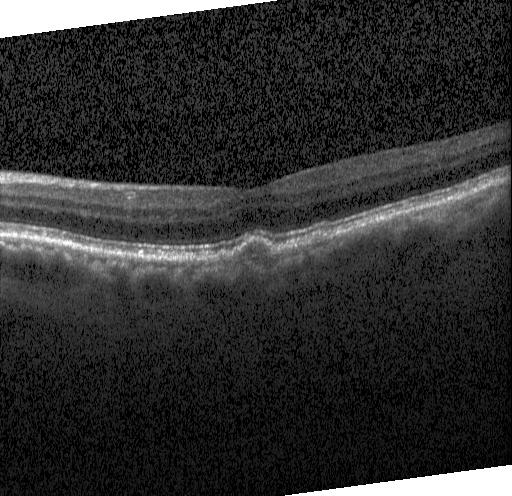 Optical coherence tomography B-scan · SD-OCT · centered on the fovea · instrument: Heidelberg Spectralis. Impression: multiple drusen.